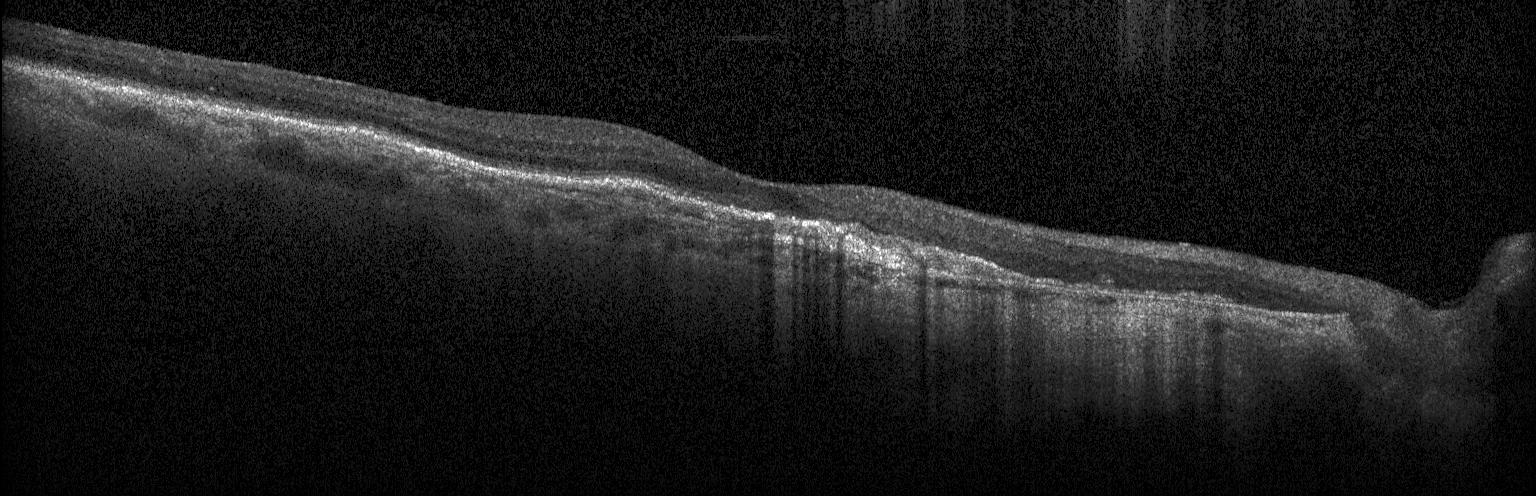 OCT B-scan · acquired on a Heidelberg Spectralis · spectral-domain optical coherence tomography · macular scan — Finding: choroidal neovascularization (CNV).